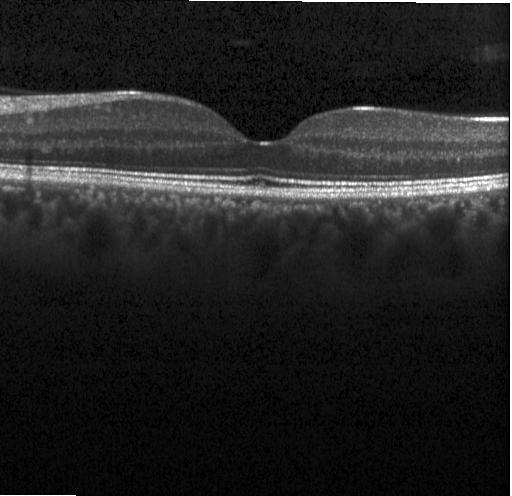 Retinal OCT B-scan.
Diagnosis: no CNV, DME, or drusen.